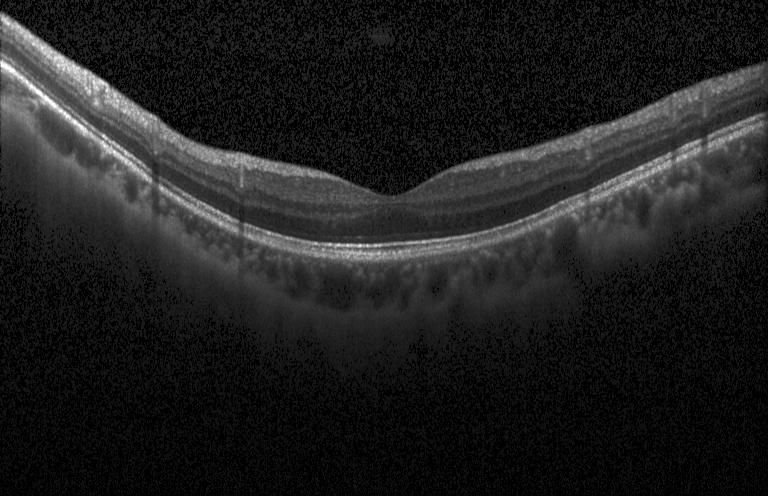 Macular OCT: no choroidal neovascularization, no diabetic macular edema, and no drusen.